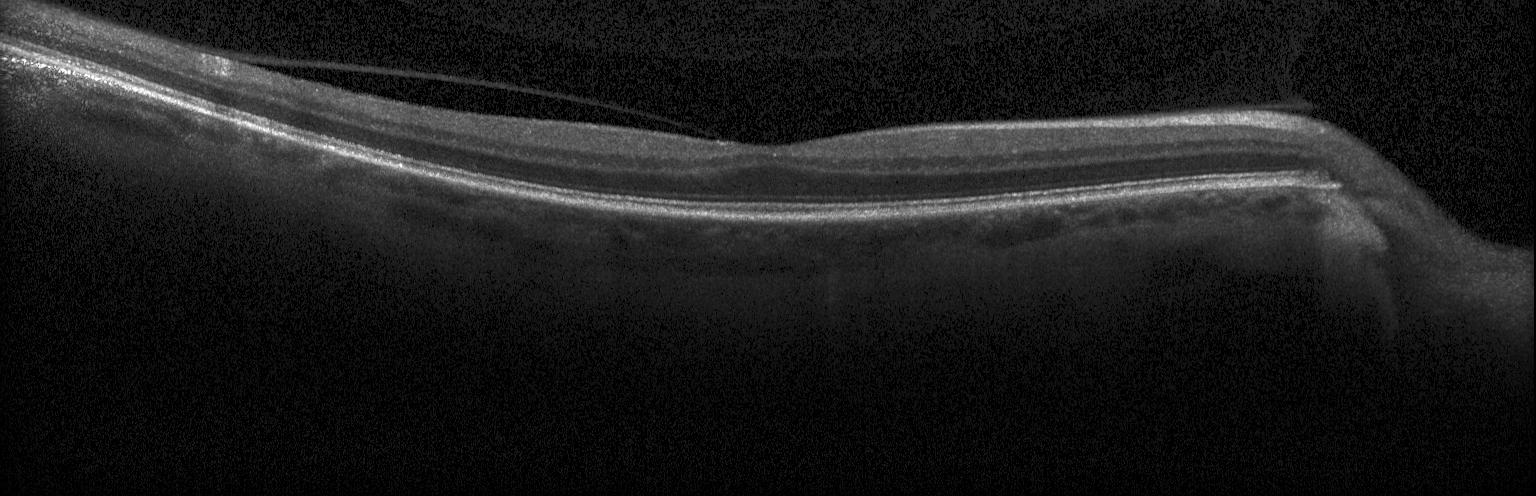 The scan shows no choroidal neovascularization, diabetic macular edema, or drusen.